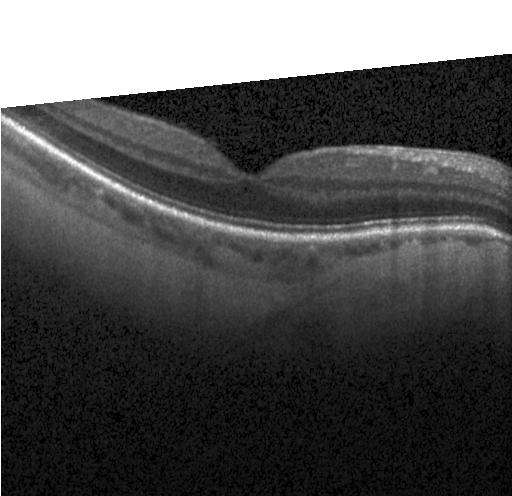
Spectral-domain optical coherence tomography, fovea-centered, OCT line scan, instrument: Heidelberg Spectralis
Diagnosis: no CNV, DME, or drusen.